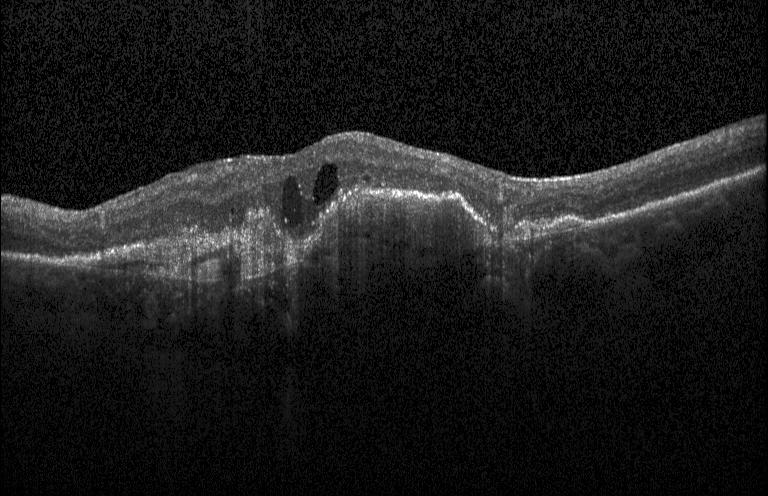
OCT scan showing a choroidal neovascular membrane.